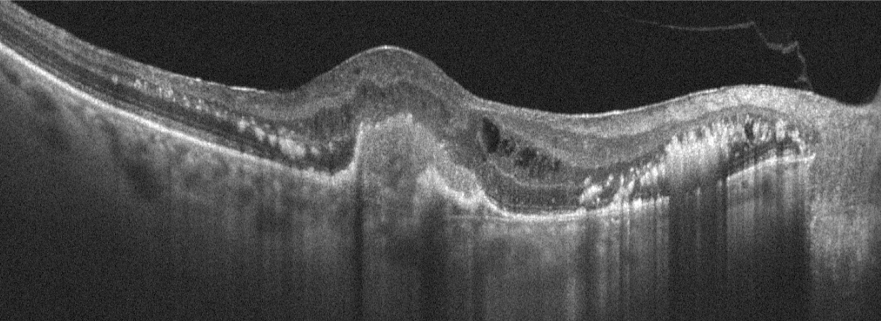 Finding: AMD.